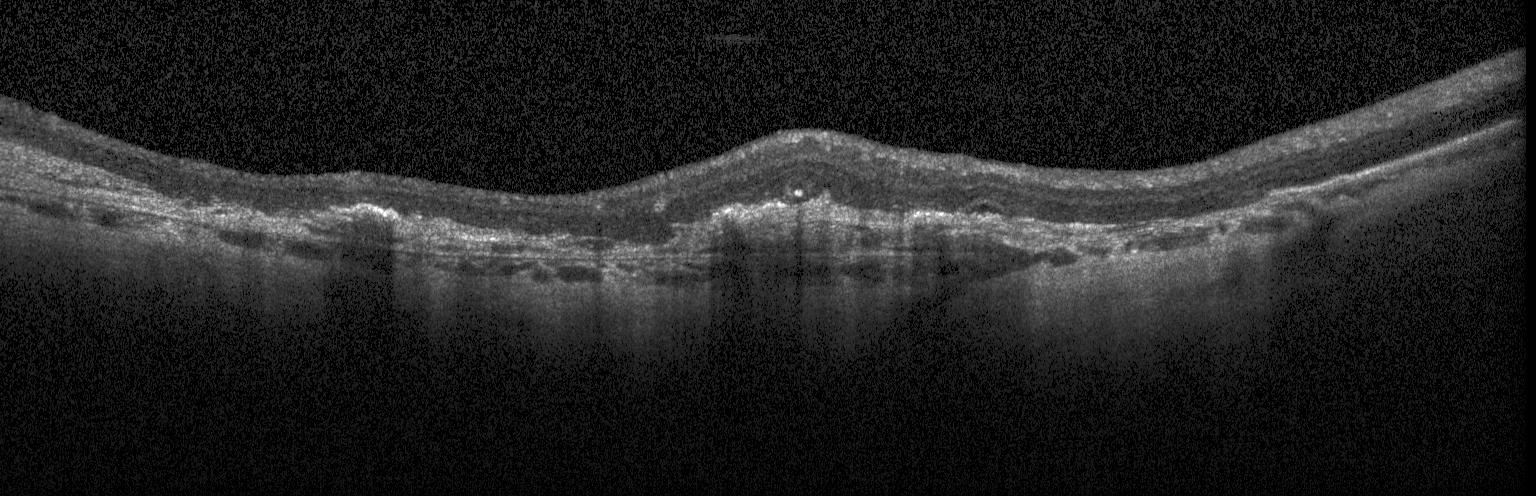 SD-OCT, OCT line scan.
Choroidal neovascularization.